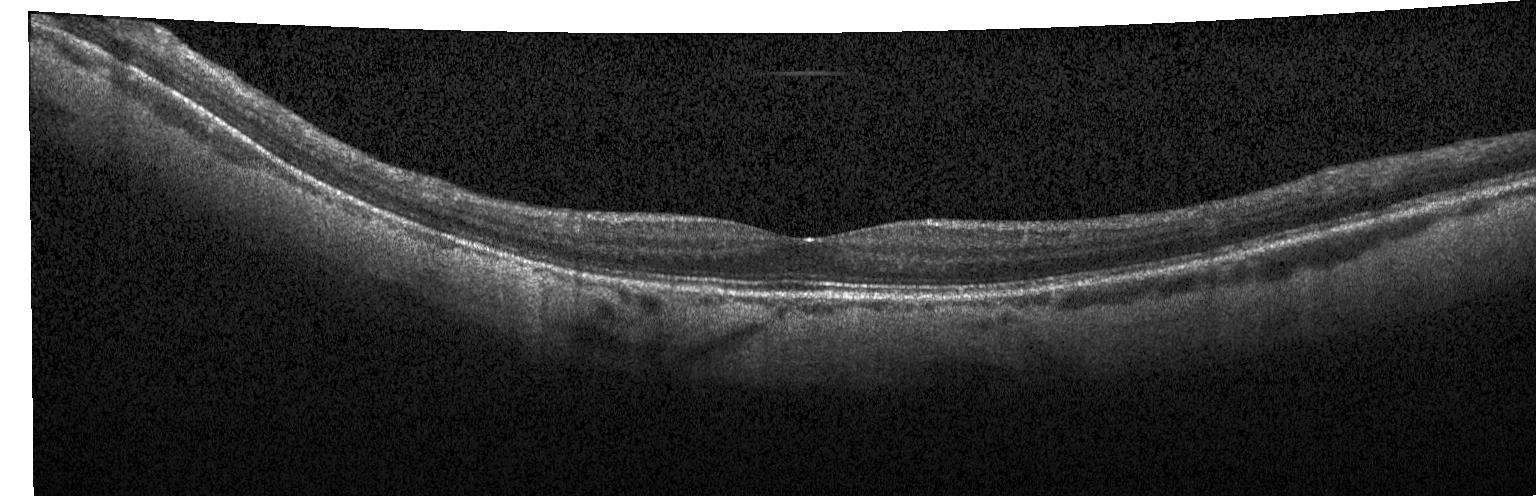

OCT B-scan showing neither CNV, DME, nor drusen.